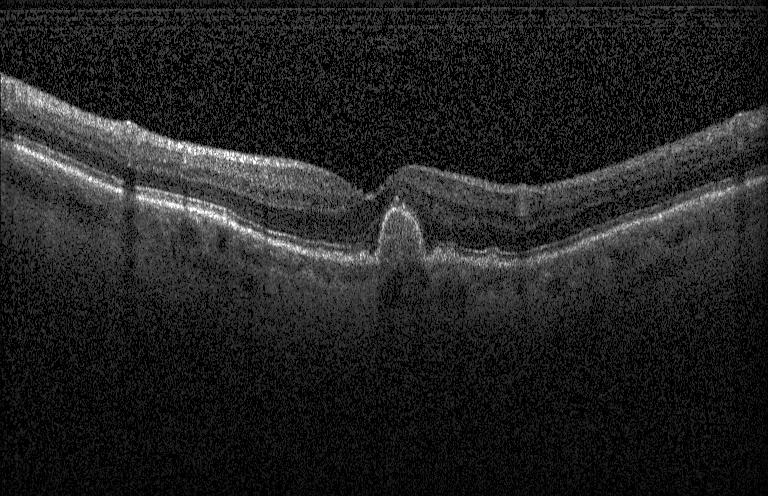 Fovea-centered; spectral-domain OCT; optical coherence tomography scan — Impression: drusen.